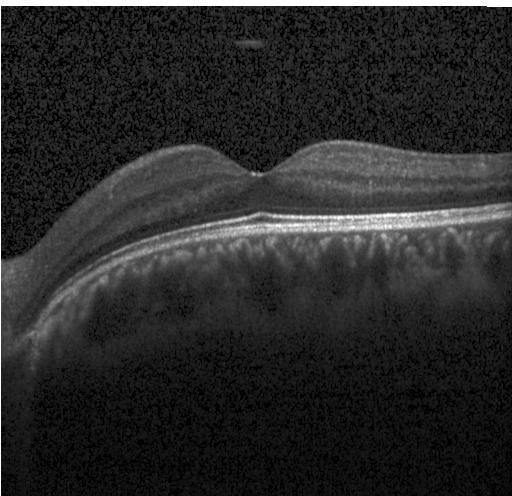

Optical coherence tomography scan
Dx: no choroidal neovascularization, diabetic macular edema, or drusen.